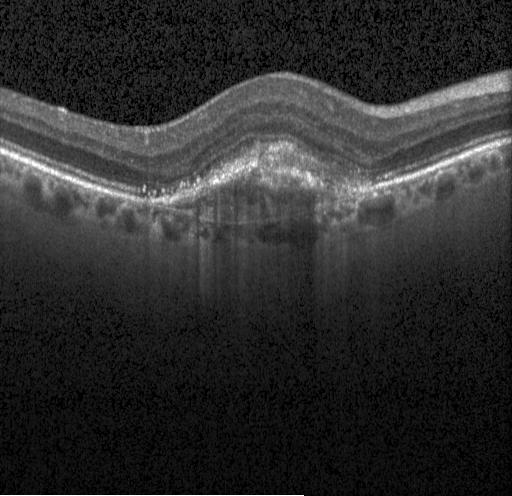 Through the macula. Heidelberg Spectralis OCT system. OCT B-scan. Spectral-domain OCT — Impression: choroidal neovascularization.